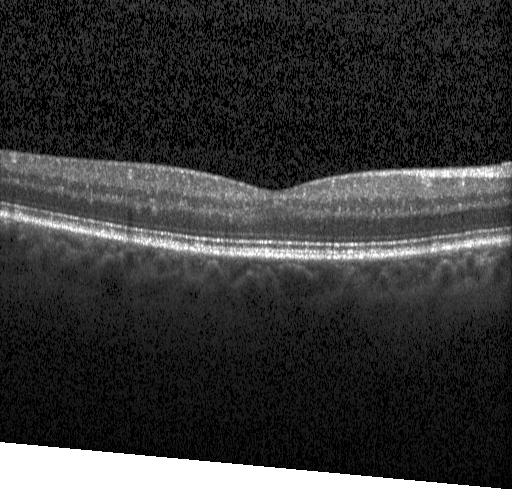

Instrument: Heidelberg Spectralis, OCT B-scan. Impression: no evidence of choroidal neovascularization, diabetic macular edema, or drusen.